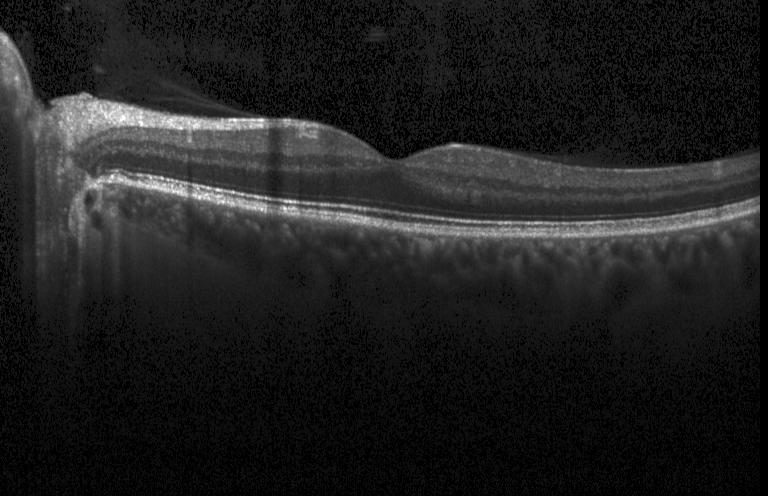 Assessment: neither choroidal neovascularization, diabetic macular edema, nor drusen.